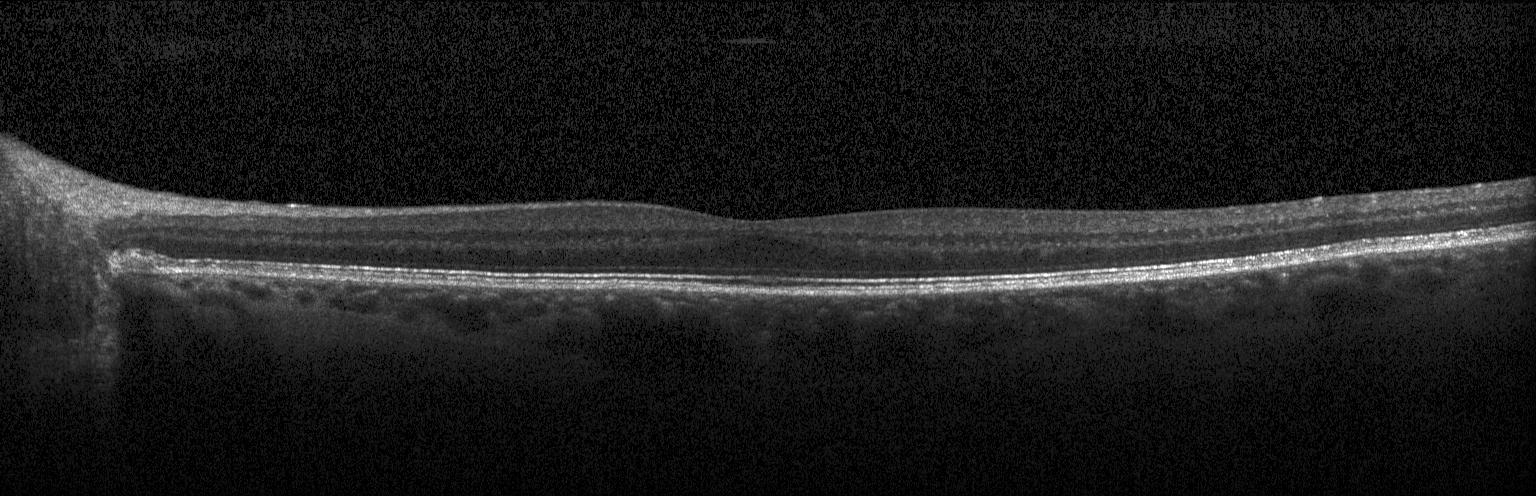 Spectral-domain OCT B-scan: neither choroidal neovascularization, diabetic macular edema, nor drusen.